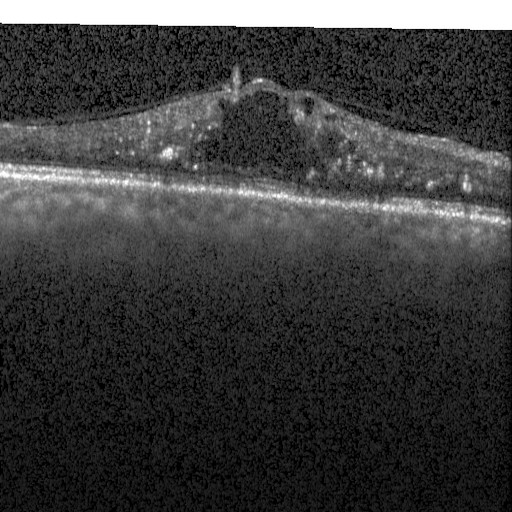 DME.